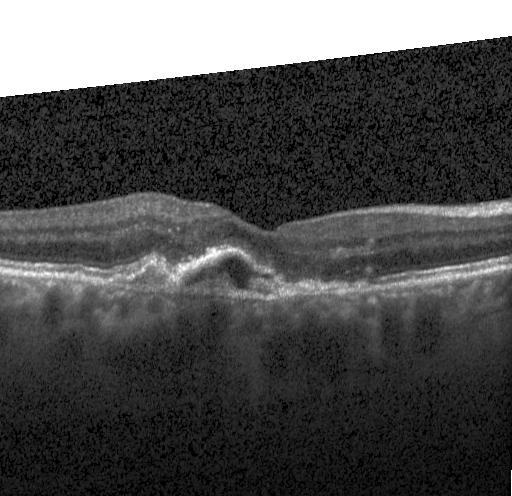

SD-OCT; horizontal scan through the fovea; optical coherence tomography scan.
Macular OCT: a choroidal neovascular membrane.